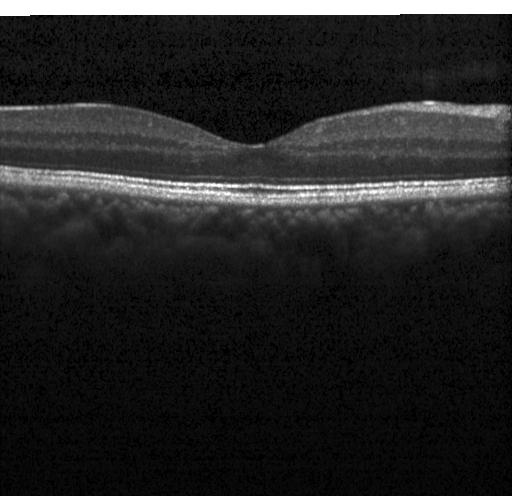 Heidelberg Spectralis. Optical coherence tomography B-scan. Horizontal scan through the fovea. Finding: neither CNV, DME, nor drusen.